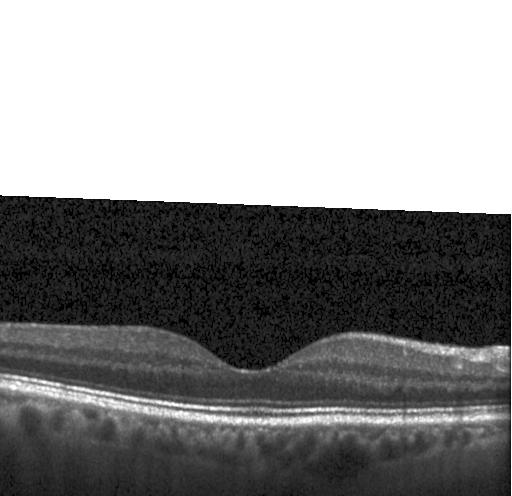

Fovea-centered, spectral-domain OCT, Heidelberg Spectralis, optical coherence tomography B-scan — Macular OCT: no choroidal neovascularization, diabetic macular edema, or drusen.